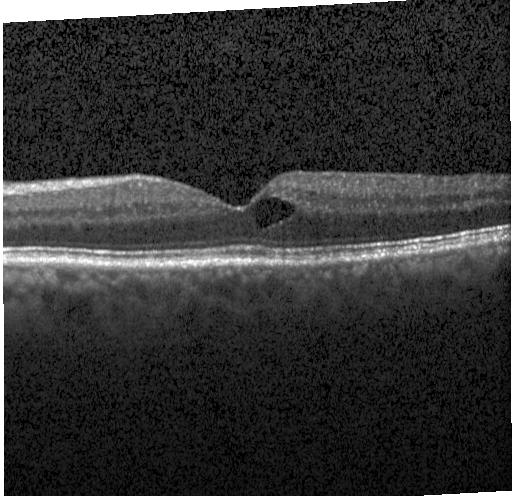

Acquired on a Heidelberg Spectralis · through the macula · retinal OCT B-scan. Impression: diabetic macular edema.